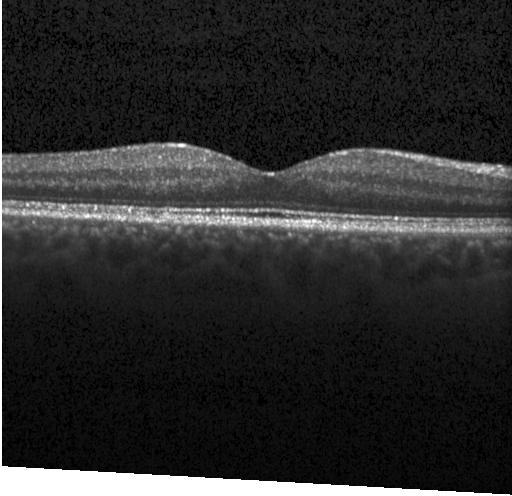
Spectral-domain optical coherence tomography · through the macula · optical coherence tomography B-scan. Finding: no choroidal neovascularization, no diabetic macular edema, and no drusen.